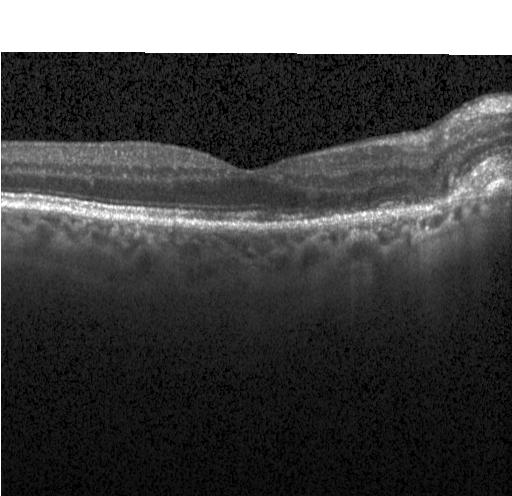
Assessment: a choroidal neovascular membrane.